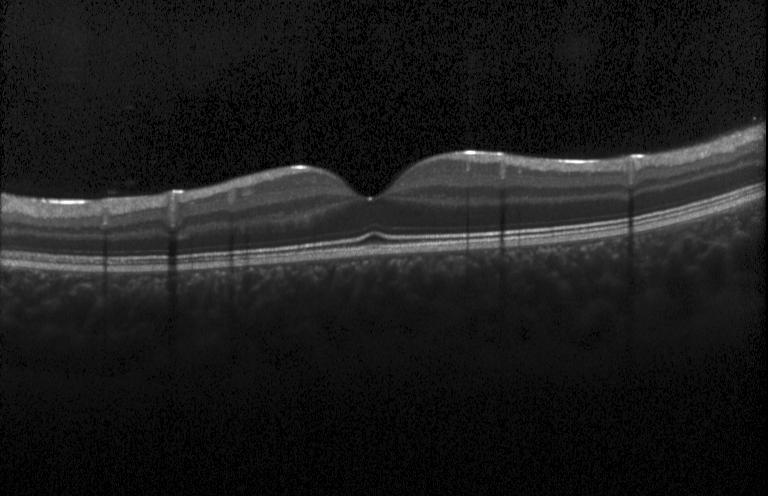
Dx: no choroidal neovascularization, no diabetic macular edema, and no drusen.